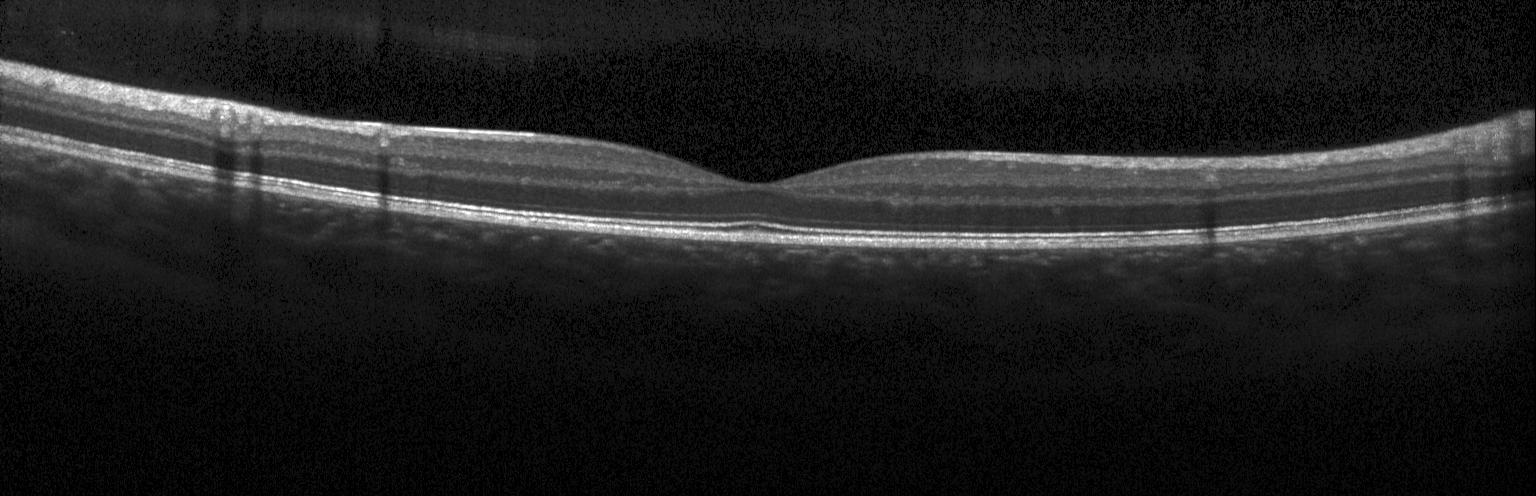
OCT B-scan, fovea-centered, SD-OCT. Diagnosis: no evidence of CNV, DME, or drusen.